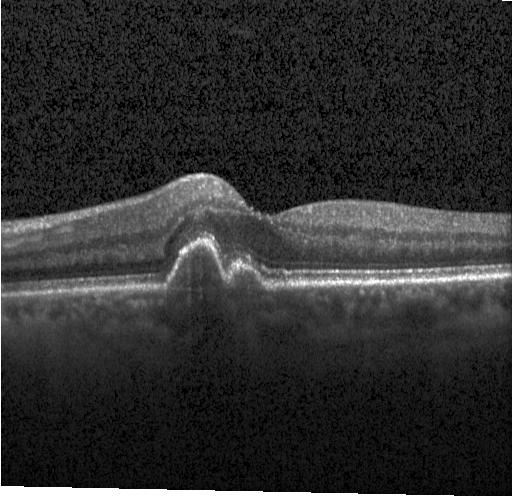
OCT line scan; centered on the fovea. The scan shows a choroidal neovascular membrane.